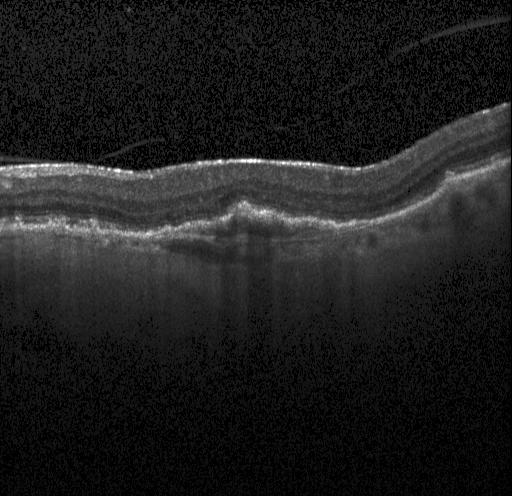
OCT scan showing CNV.